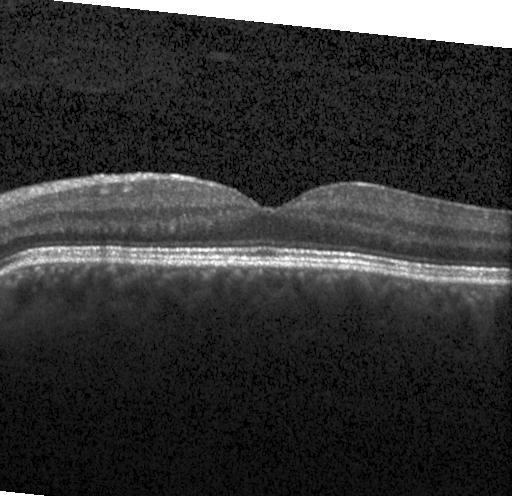 OCT line scan. Finding: no evidence of choroidal neovascularization, diabetic macular edema, or drusen.